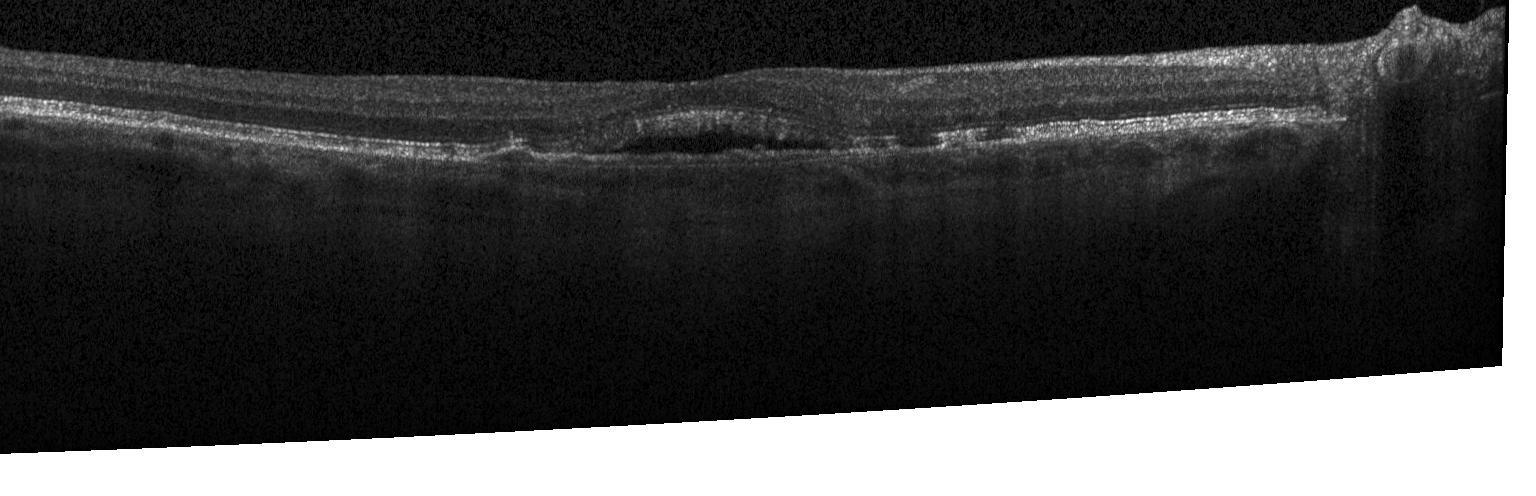 OCT line scan. OCT finding: CNV.